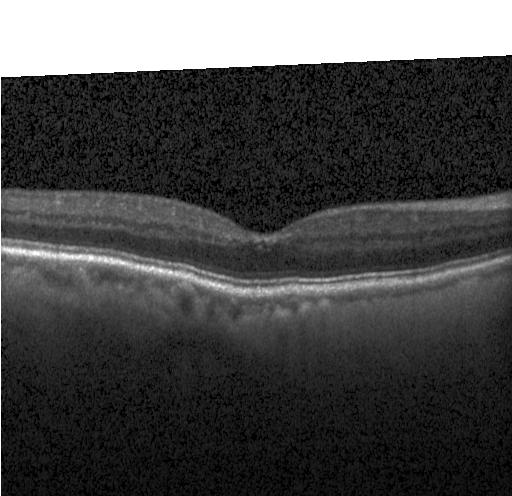

Centered on the fovea; OCT line scan; Heidelberg Spectralis
OCT finding: no CNV, DME, or drusen.